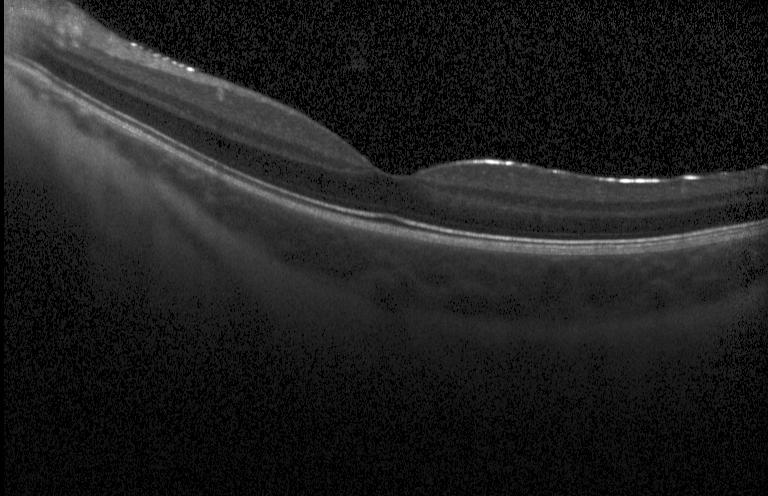

OCT finding: no choroidal neovascularization, no diabetic macular edema, and no drusen.